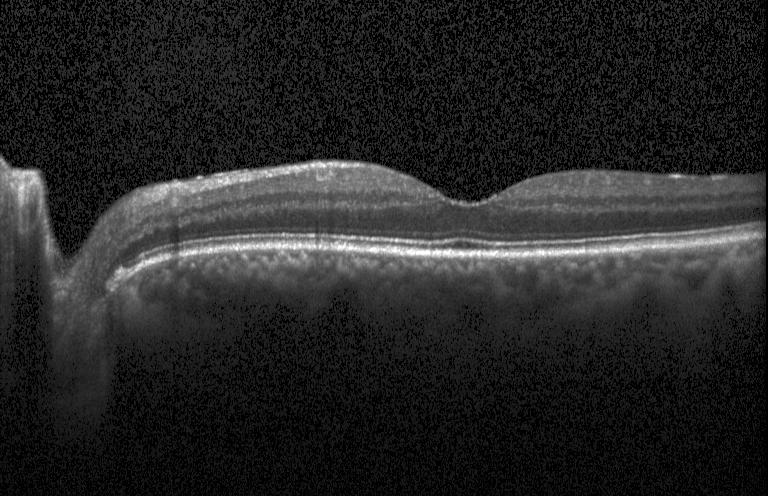
Instrument: Heidelberg Spectralis · OCT B-scan · through the macula · spectral-domain OCT
Diagnosis: no choroidal neovascularization, diabetic macular edema, or drusen.